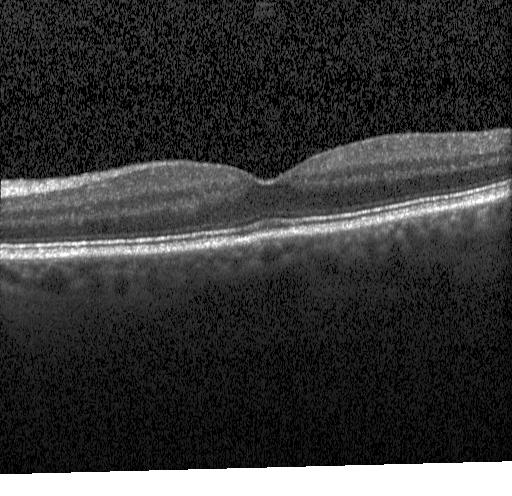
Impression: no evidence of choroidal neovascularization, diabetic macular edema, or drusen.